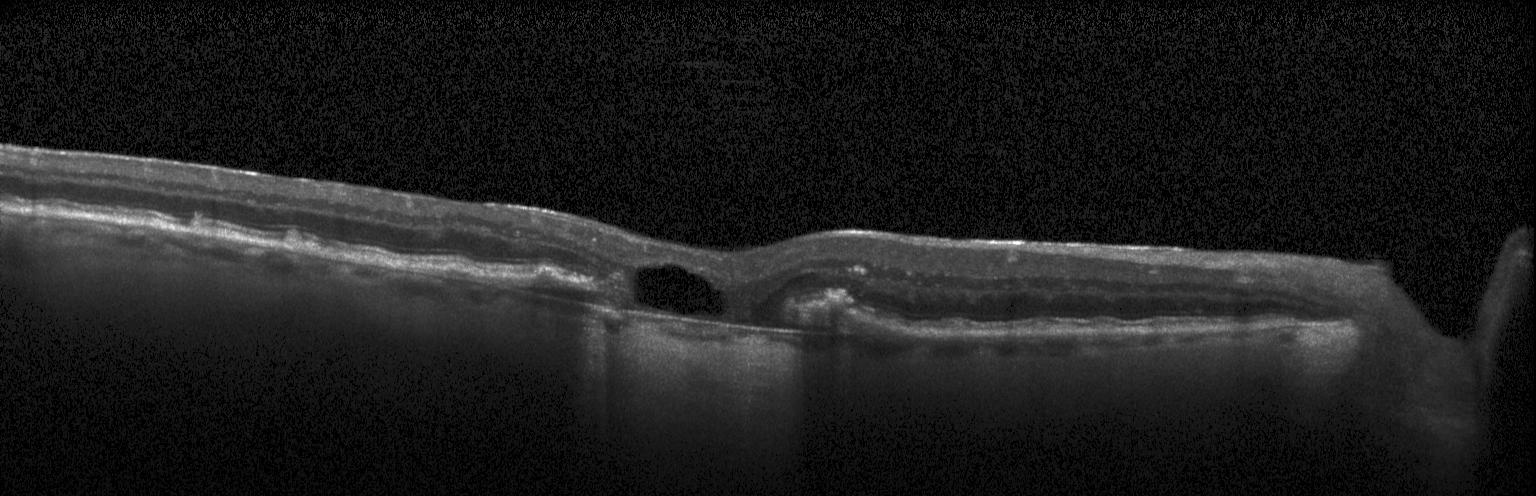
Impression: CNV.